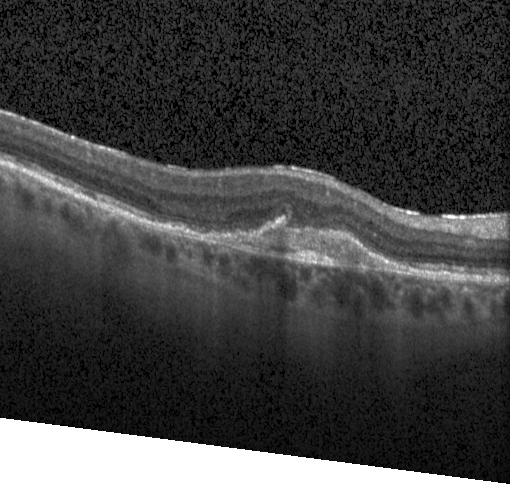

Instrument: Heidelberg Spectralis; optical coherence tomography B-scan; SD-OCT
The scan shows choroidal neovascularization (CNV).